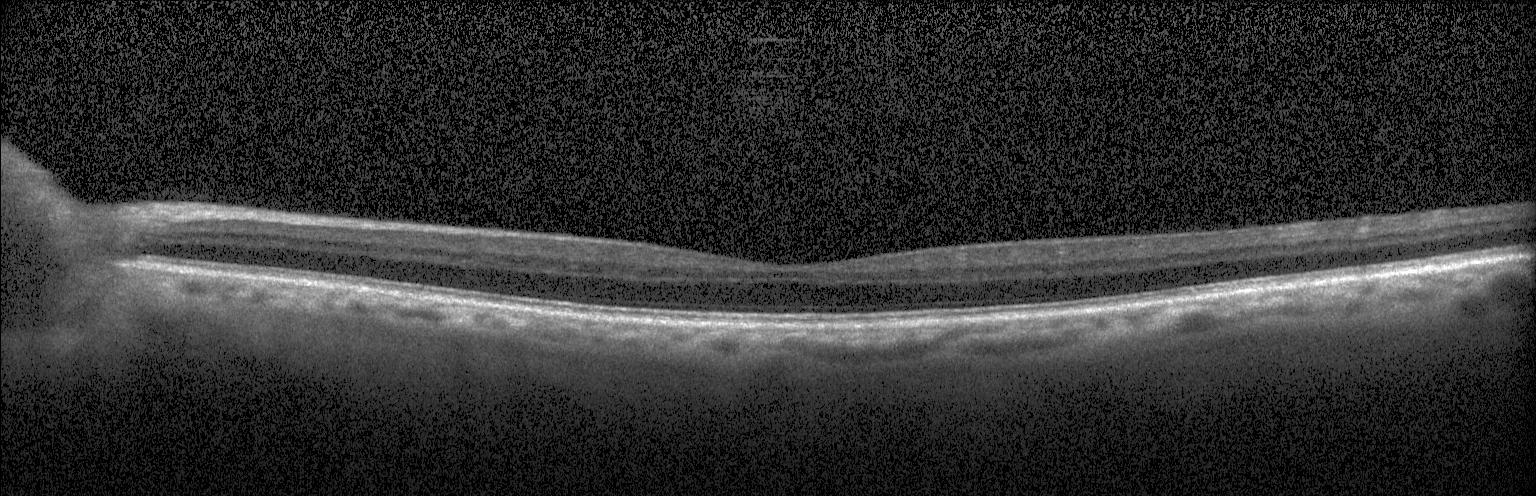

Dx: neither choroidal neovascularization, diabetic macular edema, nor drusen.